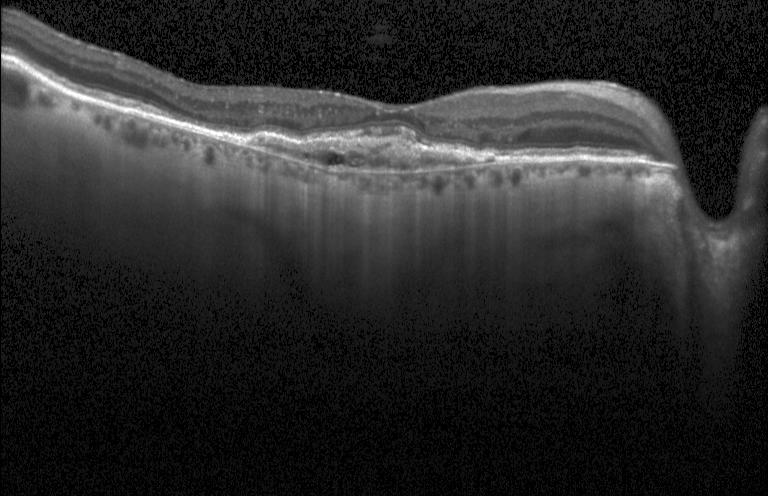
Horizontal scan through the fovea; Heidelberg Spectralis OCT system; retinal OCT cross-section; spectral-domain optical coherence tomography. The scan shows a choroidal neovascular membrane.